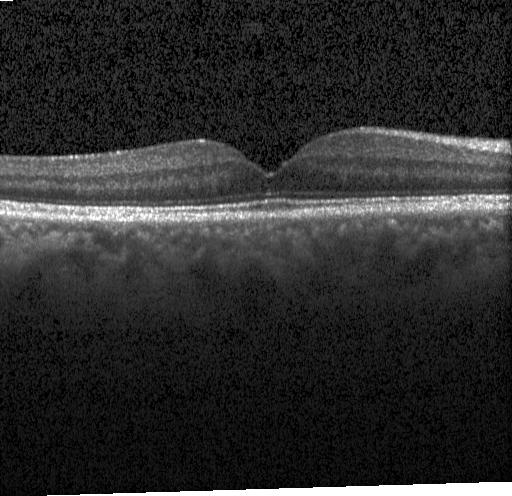
SD-OCT · optical coherence tomography scan · acquired on a Heidelberg Spectralis · fovea-centered. The scan shows no choroidal neovascularization, no diabetic macular edema, and no drusen.